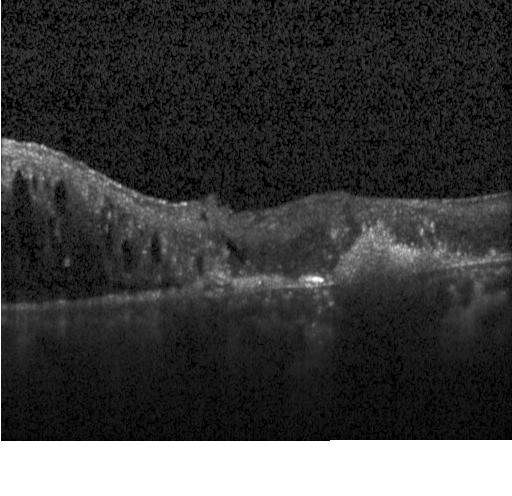 Assessment: a choroidal neovascular membrane.